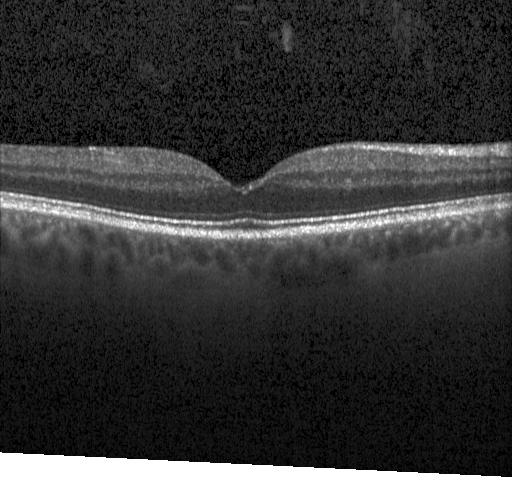

Horizontal scan through the fovea. Retinal OCT B-scan
Diagnosis: no choroidal neovascularization, diabetic macular edema, or drusen.